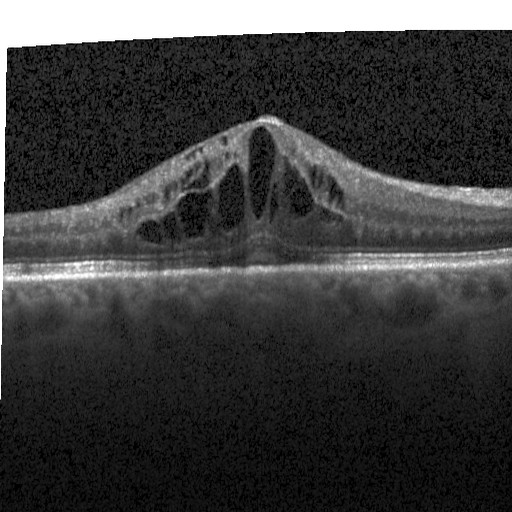

Optical coherence tomography scan. DME.